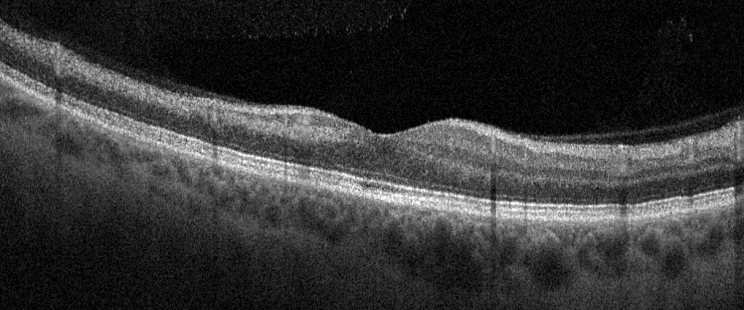

OCT B-scan. Through the macula. Acquired on an Optovue Avanti RTVue XR.
This B-scan demonstrates RVO.